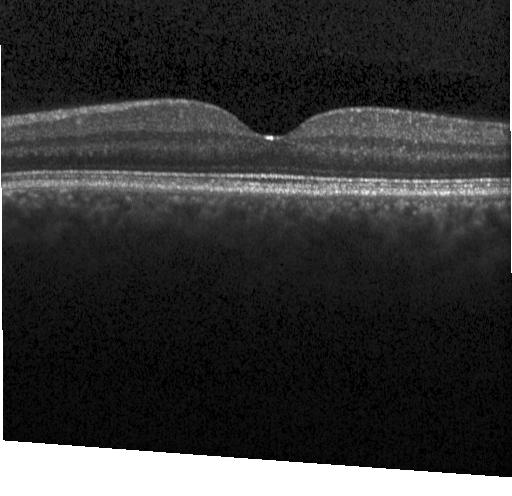 Spectral-domain OCT · centered on the fovea · Heidelberg Spectralis · OCT line scan. Finding: no CNV, no DME, and no drusen.